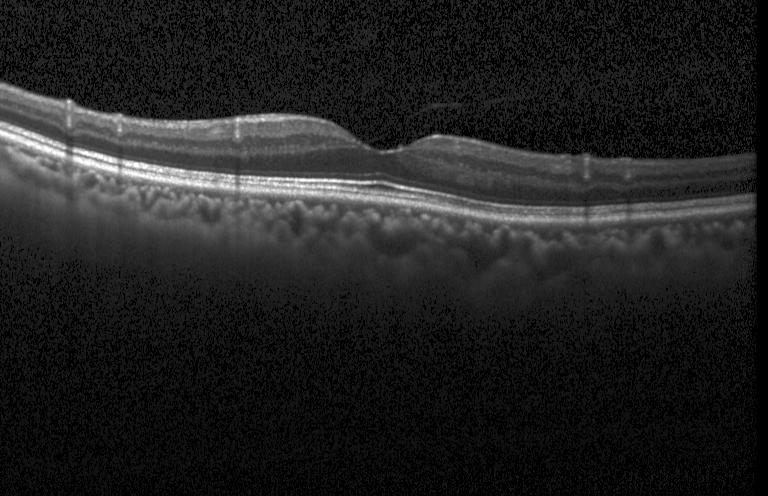
SD-OCT; retinal OCT B-scan. Assessment: no CNV, no DME, and no drusen.